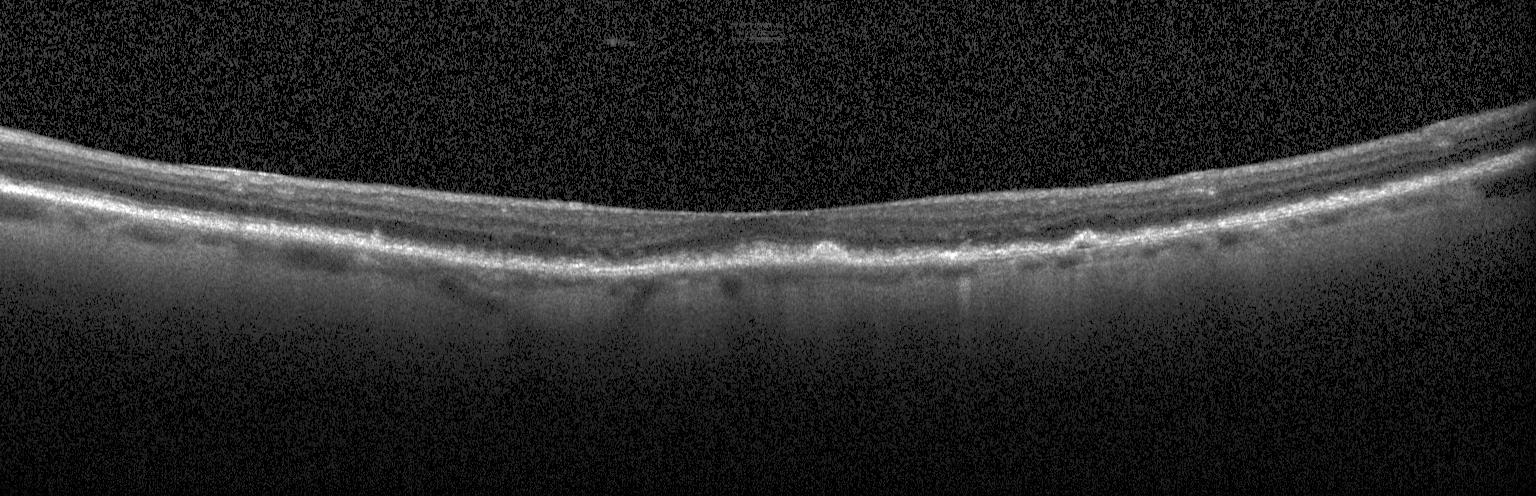 Optical coherence tomography scan, horizontal scan through the fovea. The scan shows a choroidal neovascular membrane.